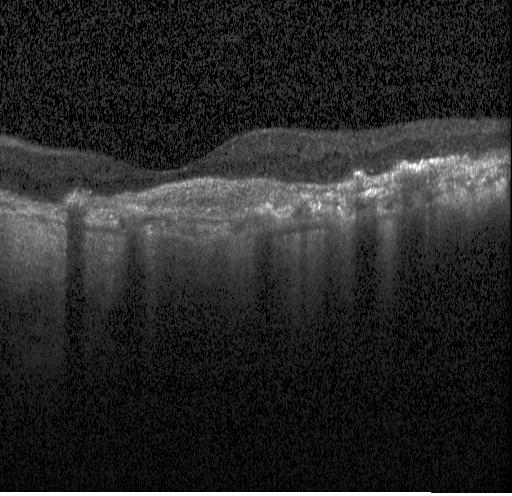 Impression: a choroidal neovascular membrane.